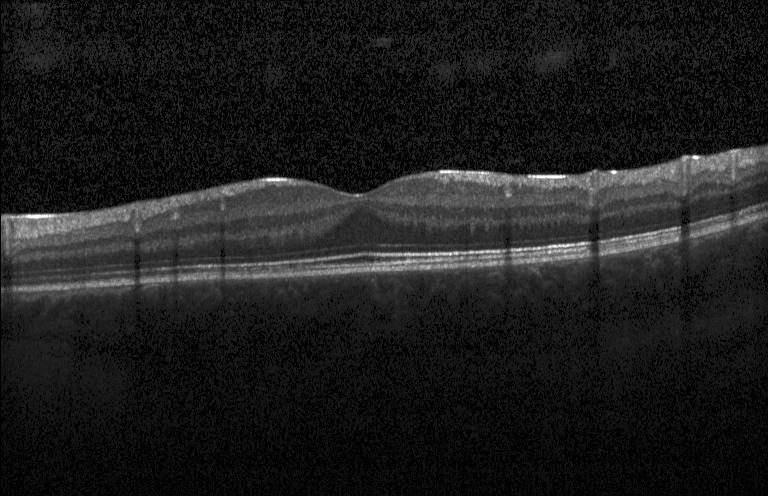

Centered on the fovea. Retinal OCT cross-section. Spectral-domain OCT
Dx: no evidence of choroidal neovascularization, diabetic macular edema, or drusen.